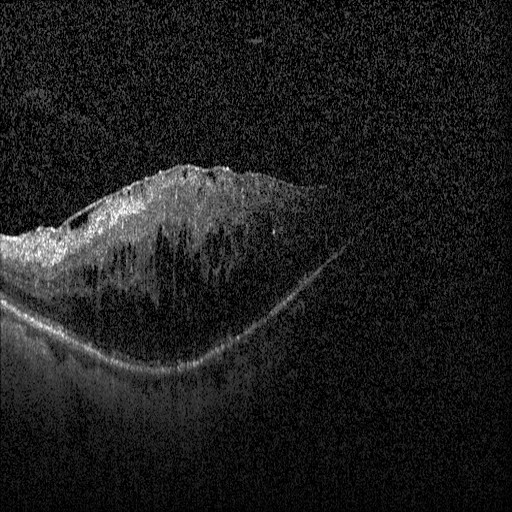

Acquired on a Heidelberg Spectralis · horizontal scan through the fovea · optical coherence tomography scan.
OCT finding: diabetic macular edema.